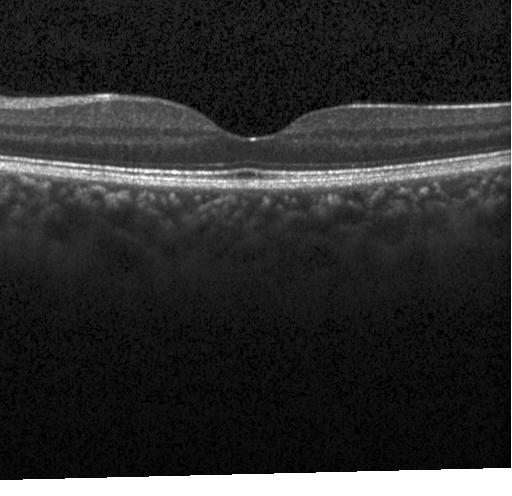

Diagnosis: neither choroidal neovascularization, diabetic macular edema, nor drusen.